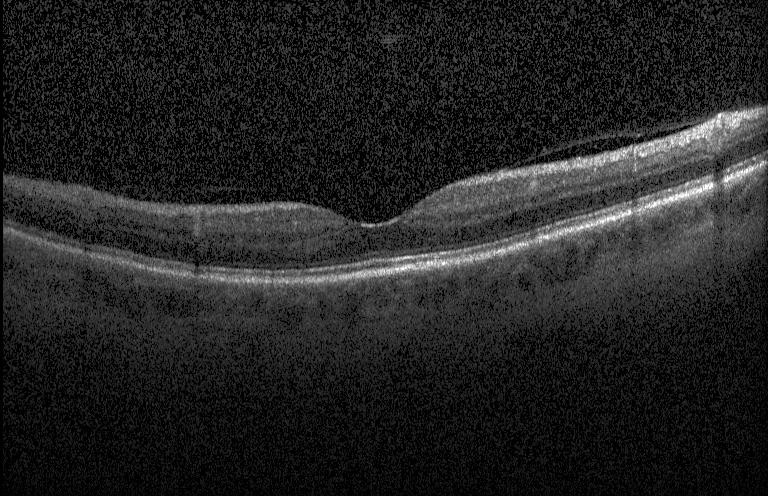
No choroidal neovascularization, no diabetic macular edema, and no drusen.